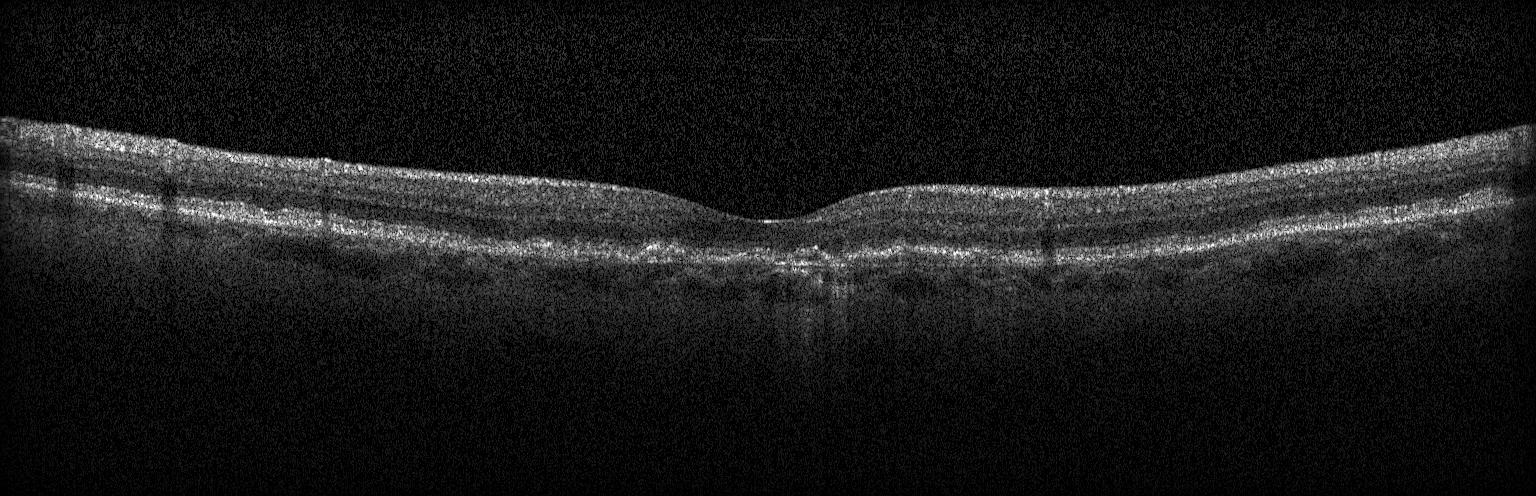 Spectral-domain OCT · Heidelberg Spectralis · optical coherence tomography scan · centered on the fovea. Finding: a choroidal neovascular membrane.